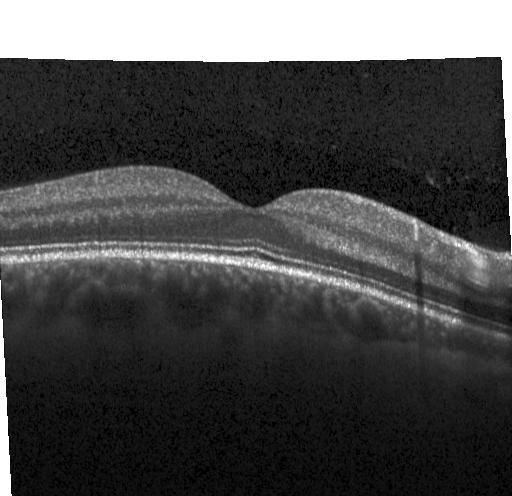

Diagnosis: no choroidal neovascularization, diabetic macular edema, or drusen.